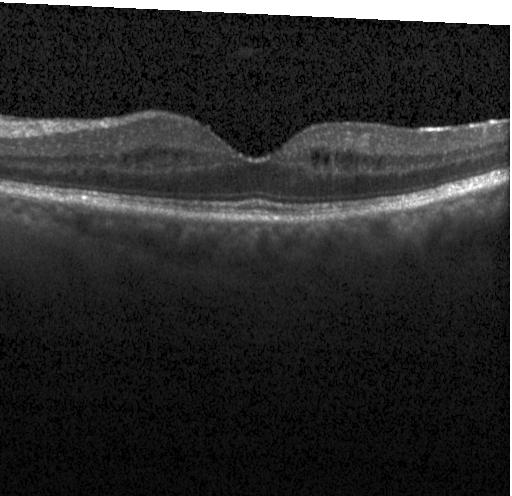
Acquired on a Heidelberg Spectralis; spectral-domain OCT; retinal OCT cross-section
Impression: DME.